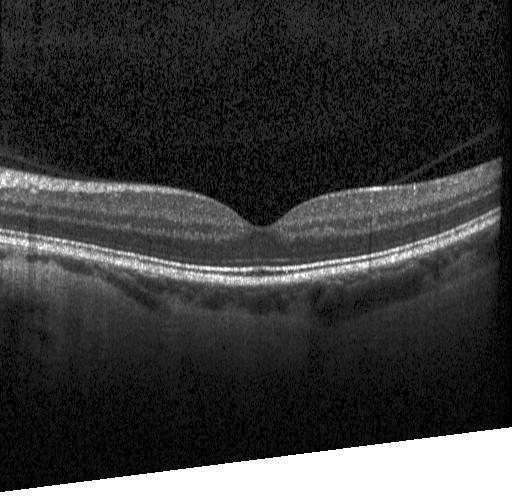
Macular OCT demonstrating no choroidal neovascularization, no diabetic macular edema, and no drusen.